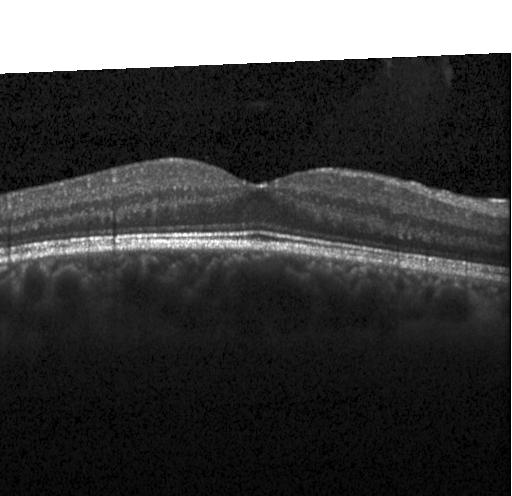

Heidelberg Spectralis. Spectral-domain OCT. Fovea-centered. OCT line scan. Assessment: no evidence of choroidal neovascularization, diabetic macular edema, or drusen.